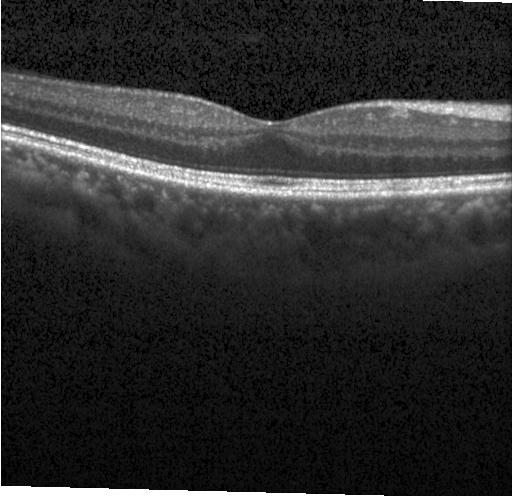 Spectral-domain OCT · Heidelberg Spectralis · optical coherence tomography B-scan
Finding: no evidence of choroidal neovascularization, diabetic macular edema, or drusen.